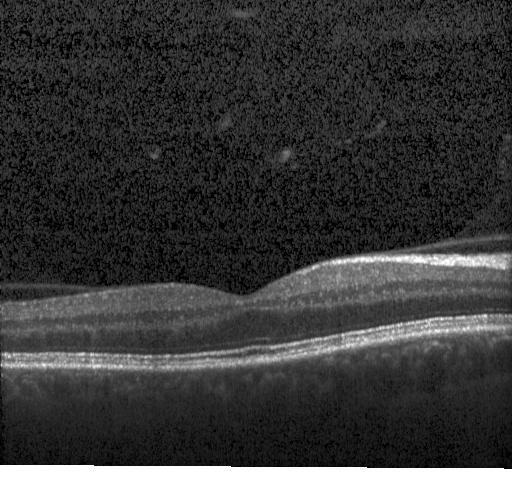

Macular scan, SD-OCT, optical coherence tomography scan, instrument: Heidelberg Spectralis. No choroidal neovascularization, no diabetic macular edema, and no drusen.